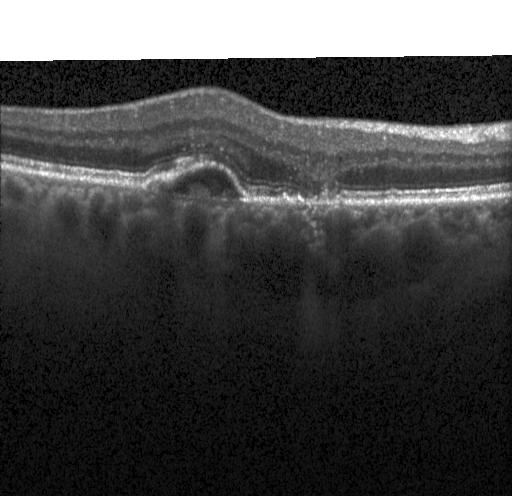
Retinal OCT cross-section
Diagnosis: a choroidal neovascular membrane.